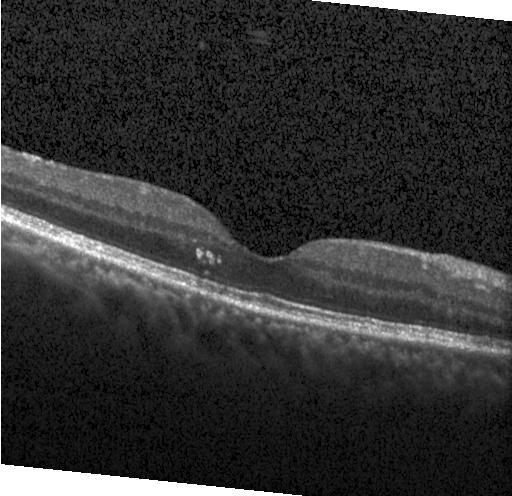
Spectral-domain OCT. Heidelberg Spectralis. Horizontal scan through the fovea. OCT B-scan — Finding: neither choroidal neovascularization, diabetic macular edema, nor drusen.